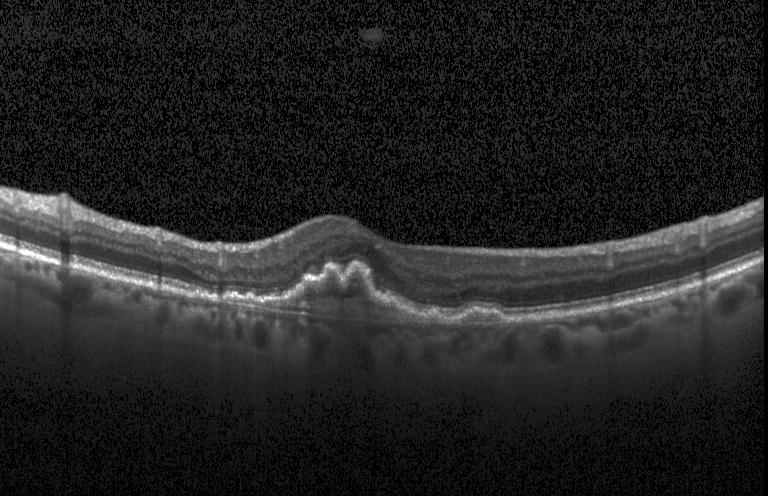
Retinal OCT cross-section. Macular OCT: CNV.